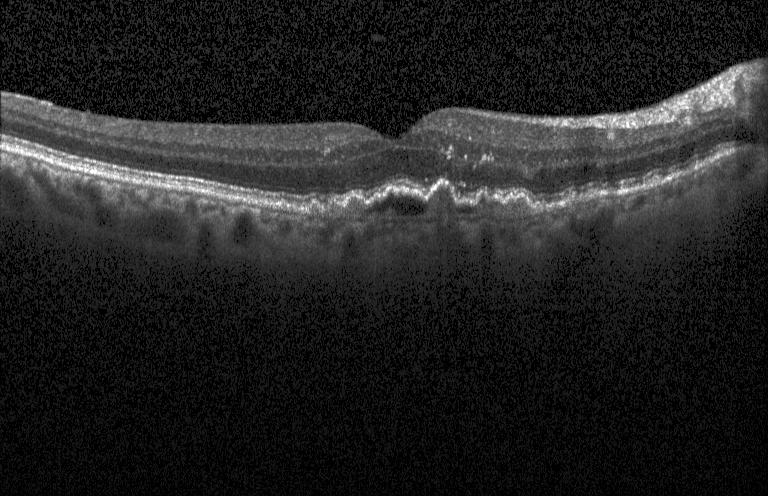 OCT B-scan
The scan shows a choroidal neovascular membrane.